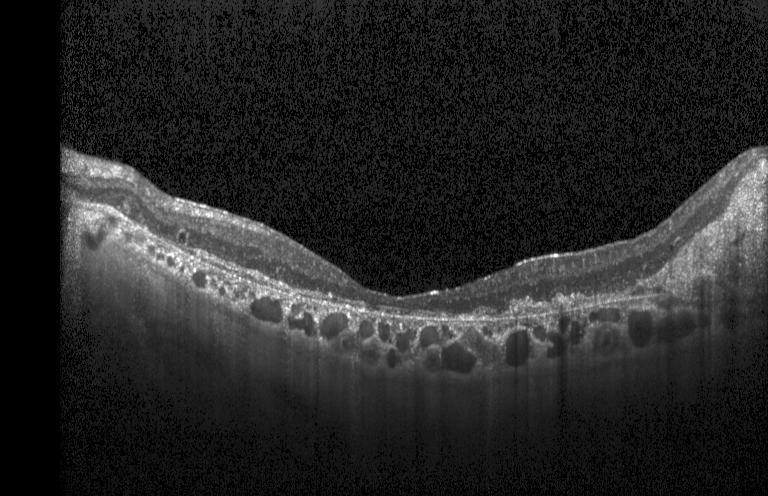 Acquired on a Heidelberg Spectralis, SD-OCT, fovea-centered, optical coherence tomography B-scan
Diagnosis: CNV.